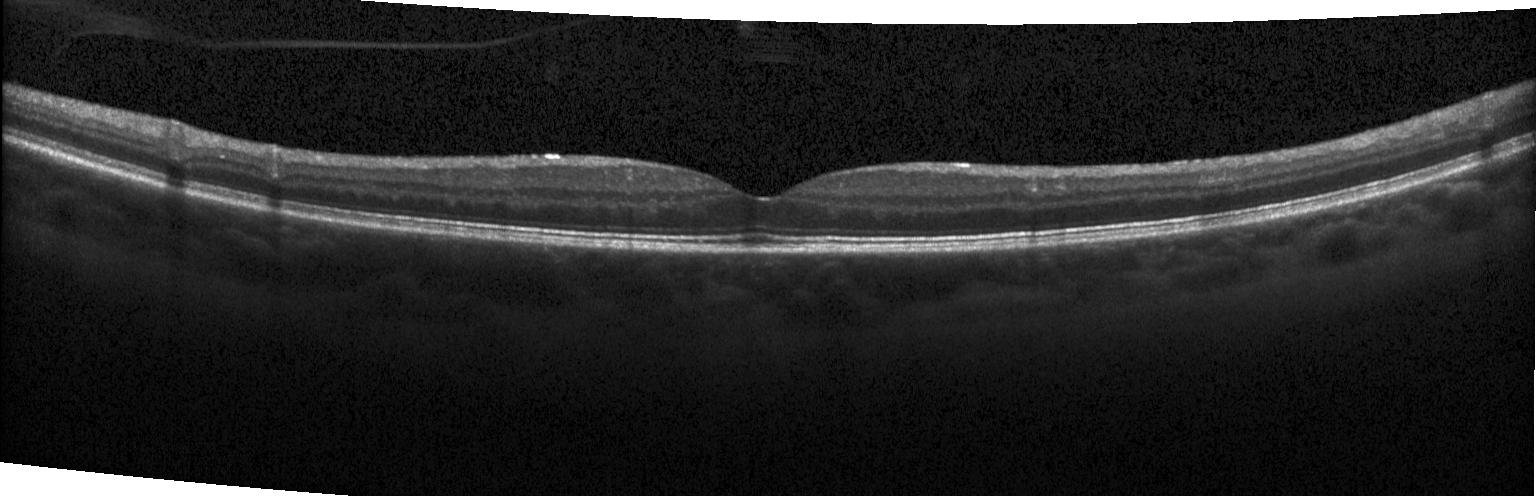

Optical coherence tomography B-scan. Assessment: no evidence of choroidal neovascularization, diabetic macular edema, or drusen.